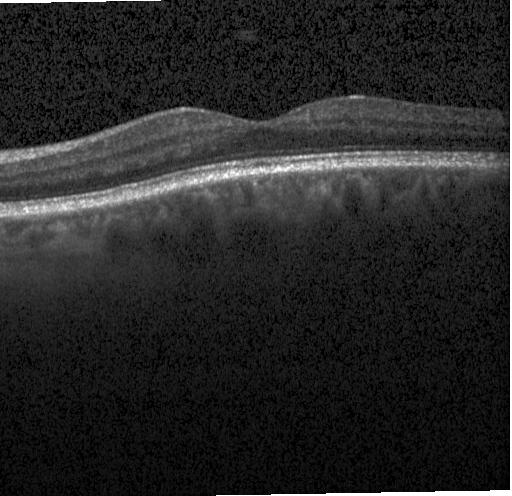
SD-OCT · acquired on a Heidelberg Spectralis · optical coherence tomography B-scan.
No choroidal neovascularization, diabetic macular edema, or drusen.